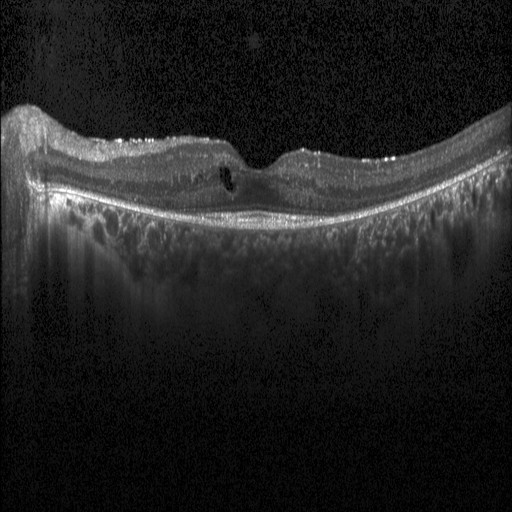 Macular OCT demonstrating diabetic macular edema.